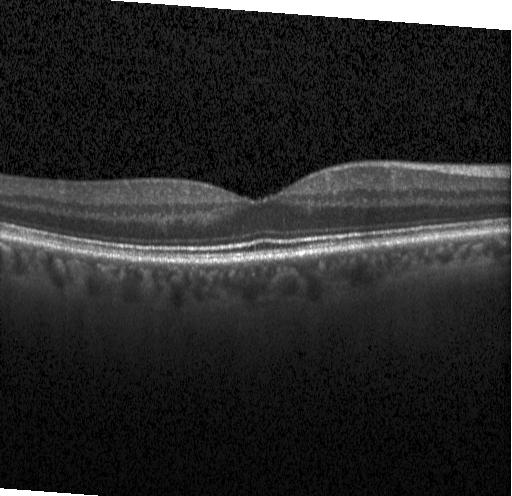

OCT B-scan · Heidelberg Spectralis OCT system · horizontal scan through the fovea · spectral-domain optical coherence tomography — Macular OCT: no evidence of choroidal neovascularization, diabetic macular edema, or drusen.